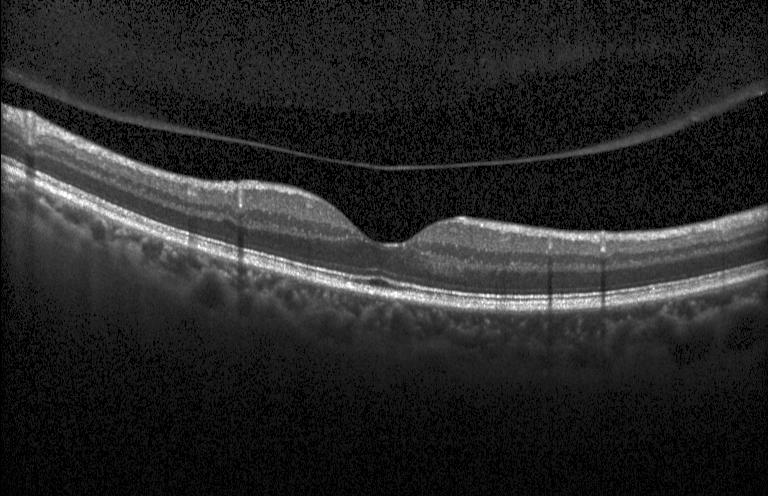 OCT line scan; SD-OCT; macular scan
Finding: no choroidal neovascularization, no diabetic macular edema, and no drusen.